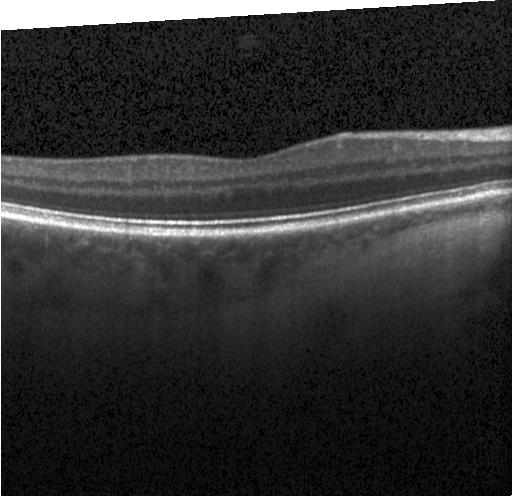 Diagnosis: neither choroidal neovascularization, diabetic macular edema, nor drusen.